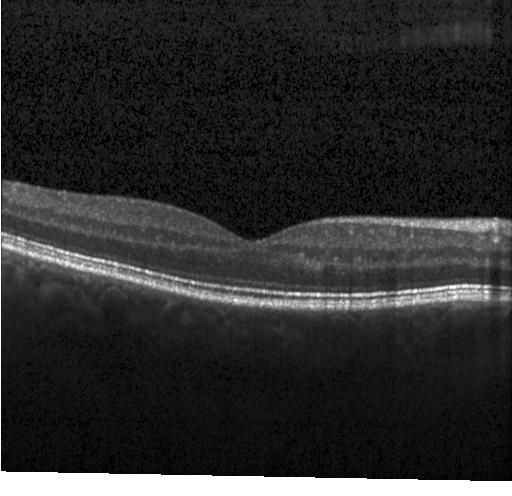 Horizontal scan through the fovea, OCT line scan, Heidelberg Spectralis, SD-OCT — The scan shows neither choroidal neovascularization, diabetic macular edema, nor drusen.